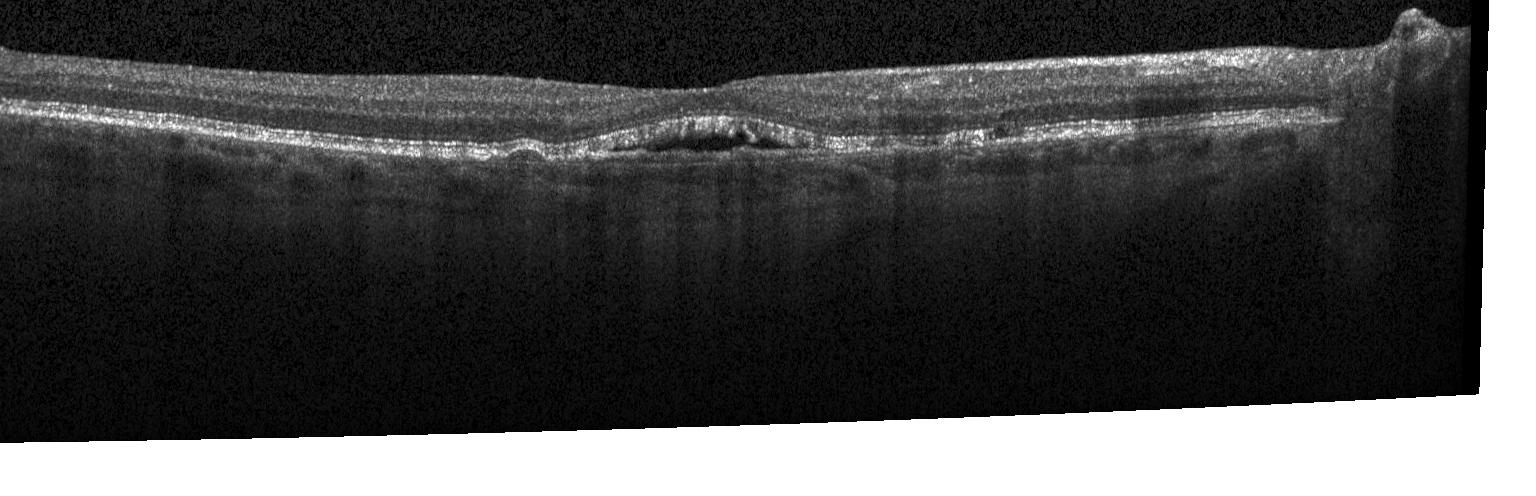 This B-scan demonstrates choroidal neovascularization (CNV).